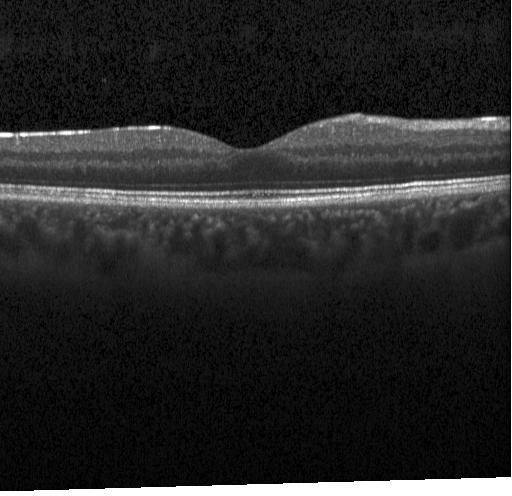 Spectral-domain optical coherence tomography · macular scan · retinal OCT cross-section.
No choroidal neovascularization, diabetic macular edema, or drusen.